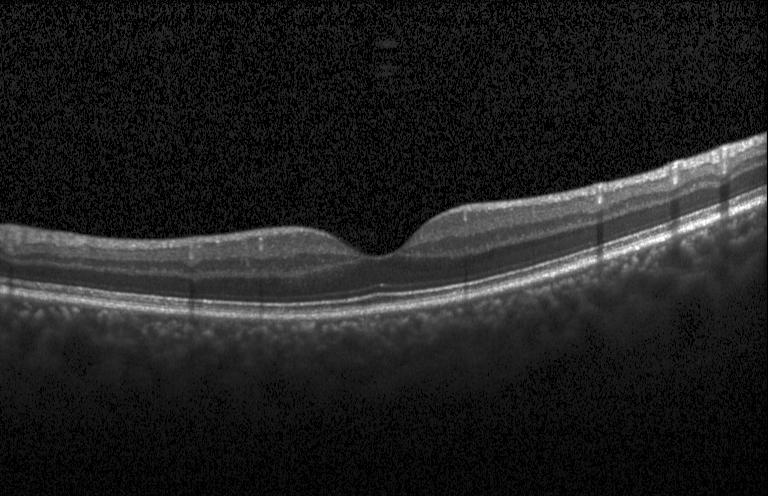

Finding: no CNV, no DME, and no drusen.